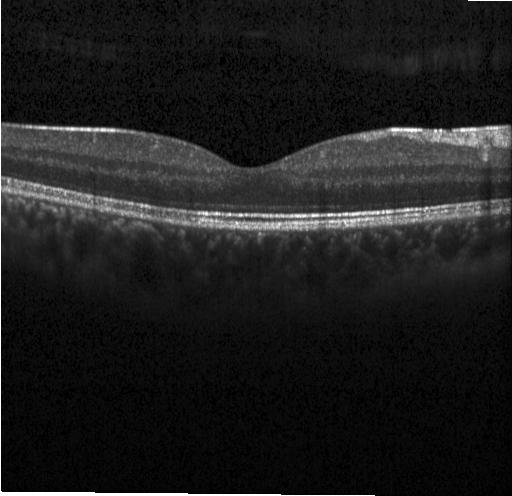
Centered on the fovea; retinal OCT B-scan; acquired on a Heidelberg Spectralis; spectral-domain optical coherence tomography
Dx: no CNV, DME, or drusen.